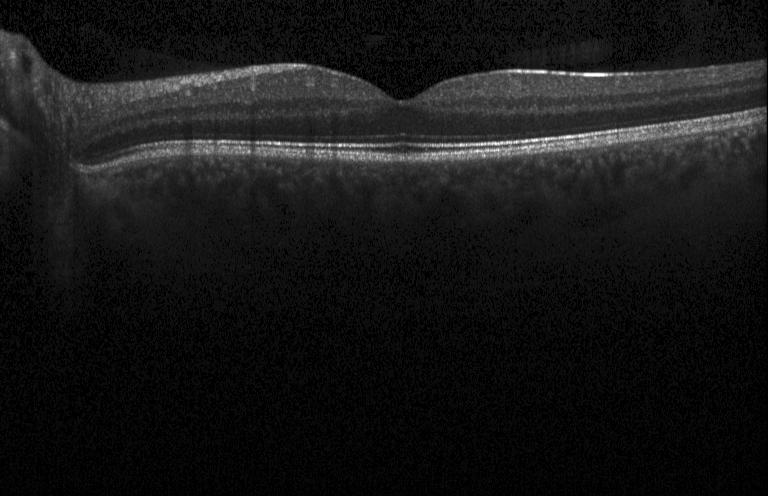 Dx: no evidence of choroidal neovascularization, diabetic macular edema, or drusen.